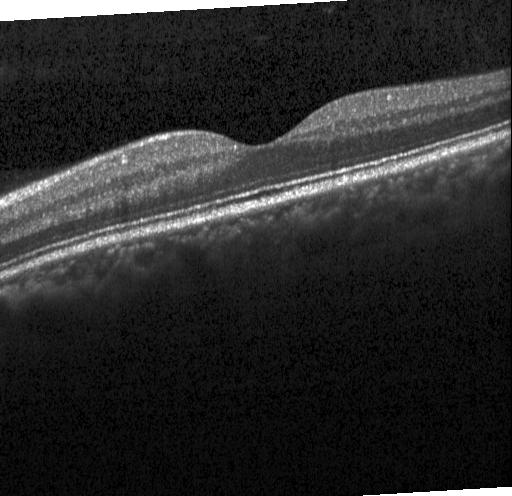 Finding: no choroidal neovascularization, diabetic macular edema, or drusen.